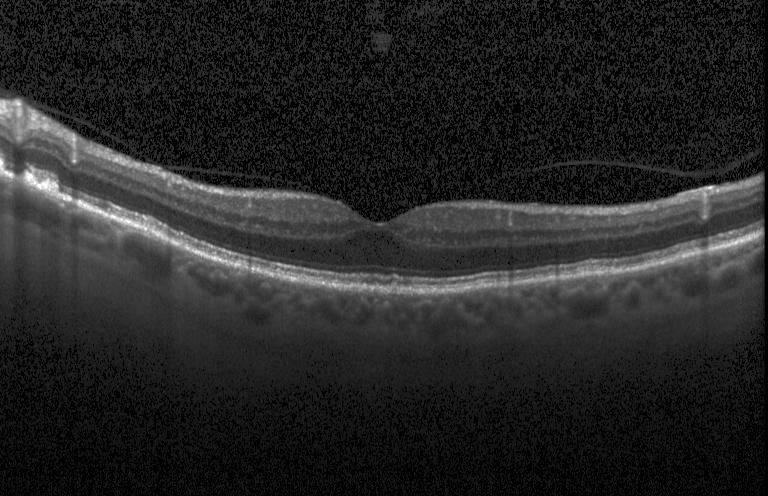
Retinal OCT cross-section; Heidelberg Spectralis OCT system; SD-OCT. Impression: neither choroidal neovascularization, diabetic macular edema, nor drusen.